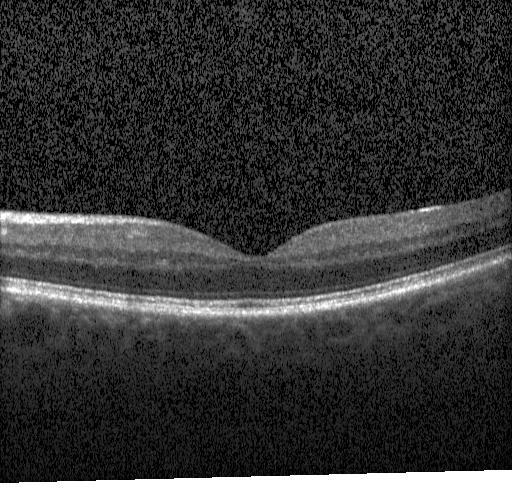

The scan shows no CNV, DME, or drusen.